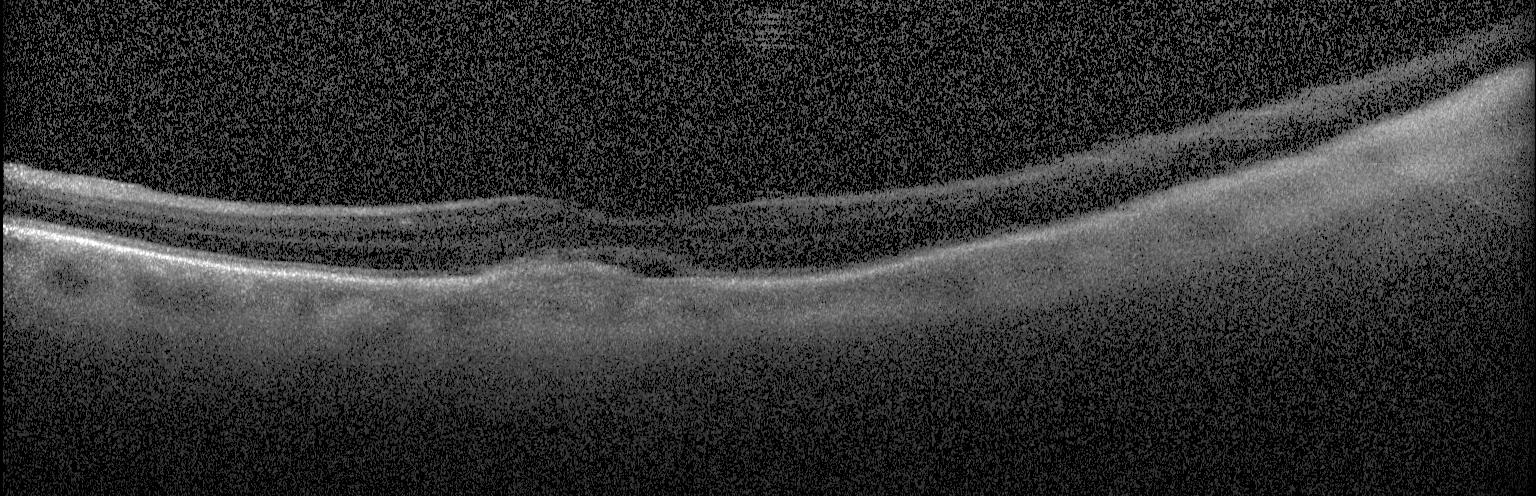 Retinal OCT cross-section · Heidelberg Spectralis
This B-scan demonstrates choroidal neovascularization.